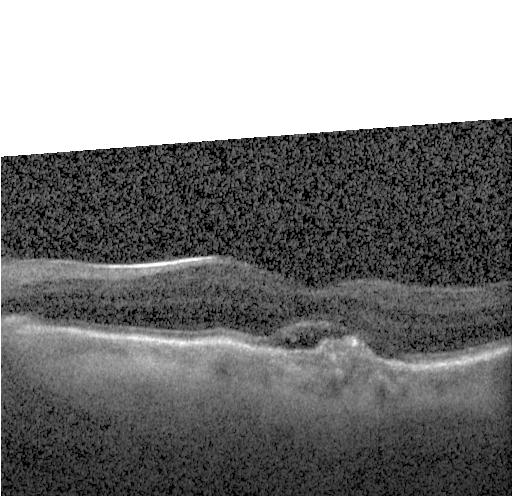

Spectral-domain OCT B-scan: choroidal neovascularization (CNV).